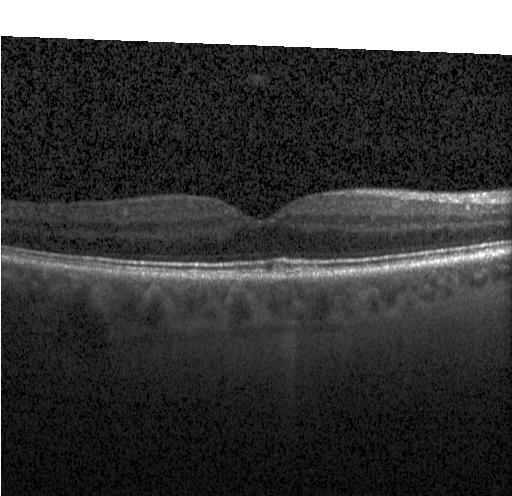

Instrument: Heidelberg Spectralis · SD-OCT · OCT B-scan · horizontal scan through the fovea. Finding: no choroidal neovascularization, no diabetic macular edema, and no drusen.